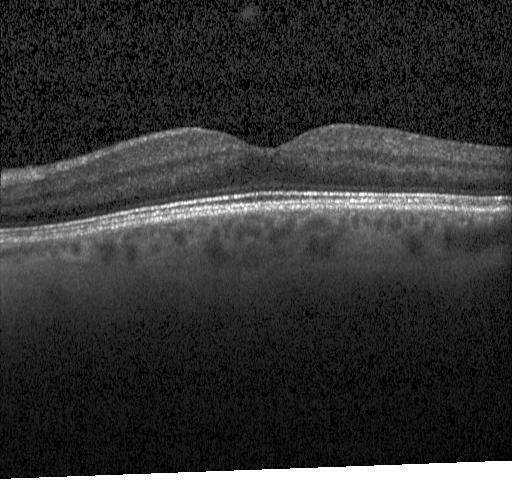 Optical coherence tomography B-scan.
Impression: no choroidal neovascularization, no diabetic macular edema, and no drusen.